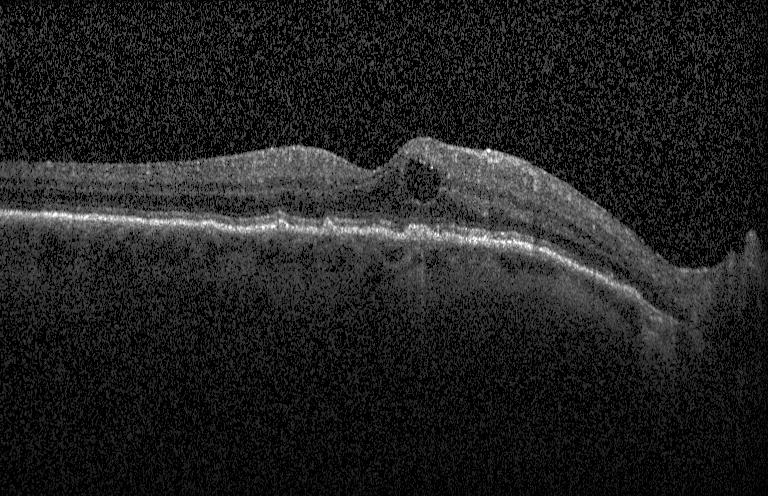
Macular scan. Retinal OCT cross-section
Finding: a choroidal neovascular membrane.